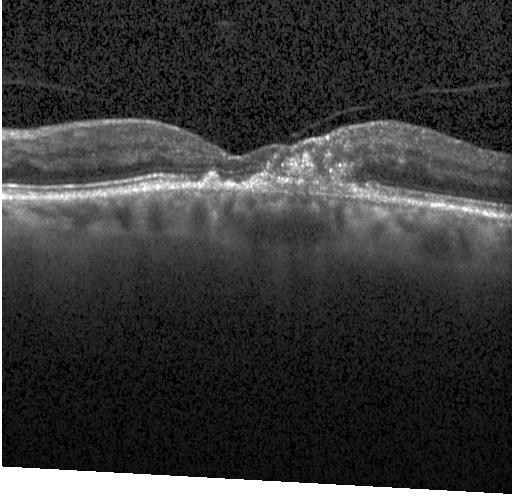
Macular scan. Retinal OCT B-scan. Spectral-domain optical coherence tomography — Impression: choroidal neovascularization.